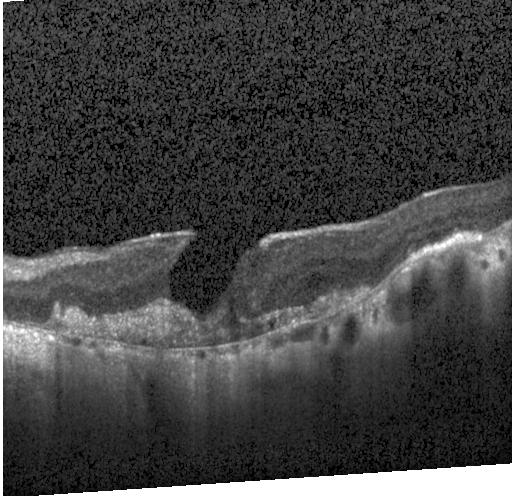 Instrument: Heidelberg Spectralis, spectral-domain OCT, through the macula, OCT line scan
Dx: CNV.